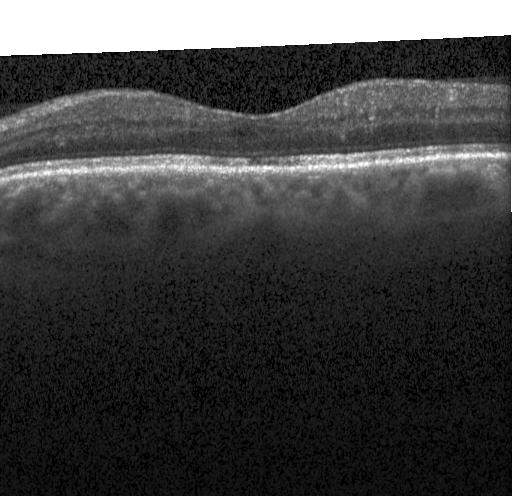 OCT B-scan · acquired on a Heidelberg Spectralis — Impression: no choroidal neovascularization, no diabetic macular edema, and no drusen.